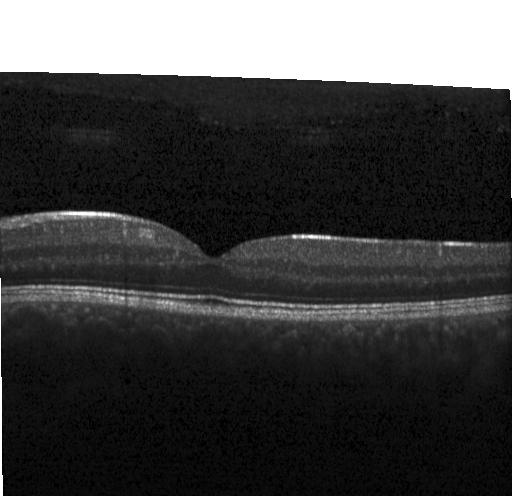

Acquired on a Heidelberg Spectralis · OCT B-scan — Impression: no evidence of CNV, DME, or drusen.